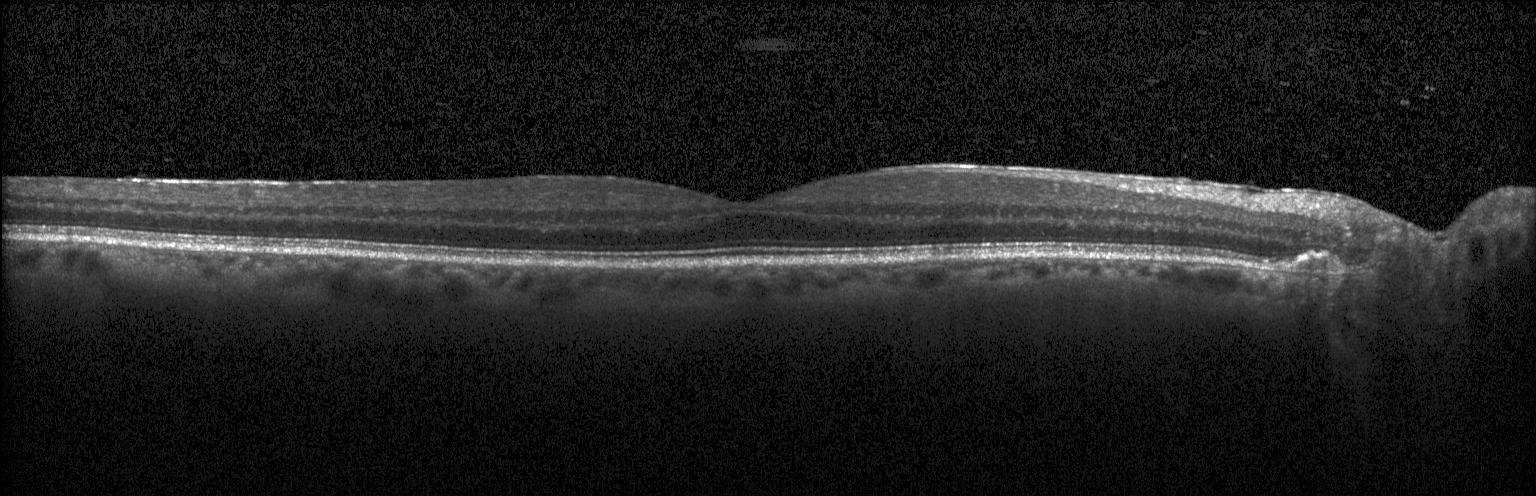 Heidelberg Spectralis OCT system, OCT B-scan — Finding: neither choroidal neovascularization, diabetic macular edema, nor drusen.